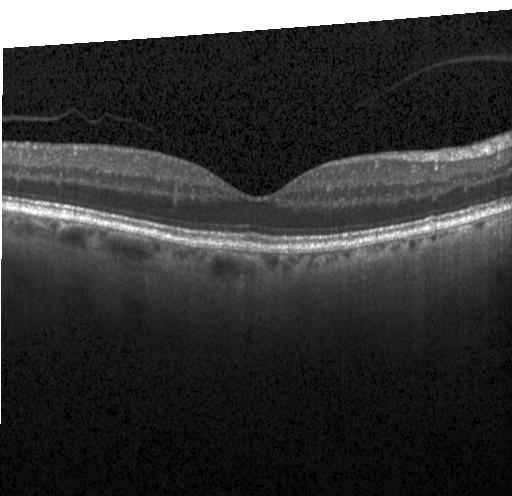

Optical coherence tomography B-scan; fovea-centered; spectral-domain optical coherence tomography.
Dx: neither CNV, DME, nor drusen.